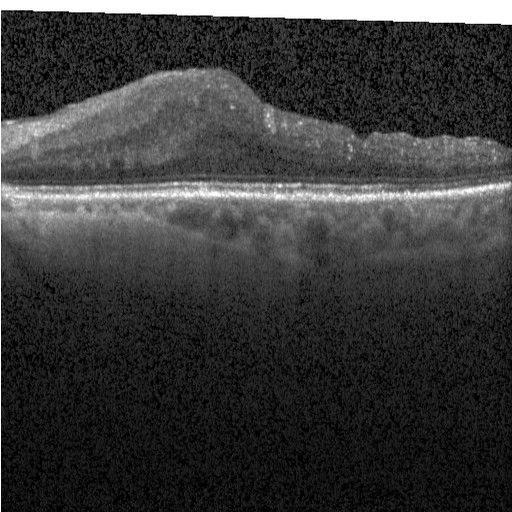 Acquired on a Heidelberg Spectralis; OCT B-scan; macular scan — Diagnosis: diabetic macular edema (DME).